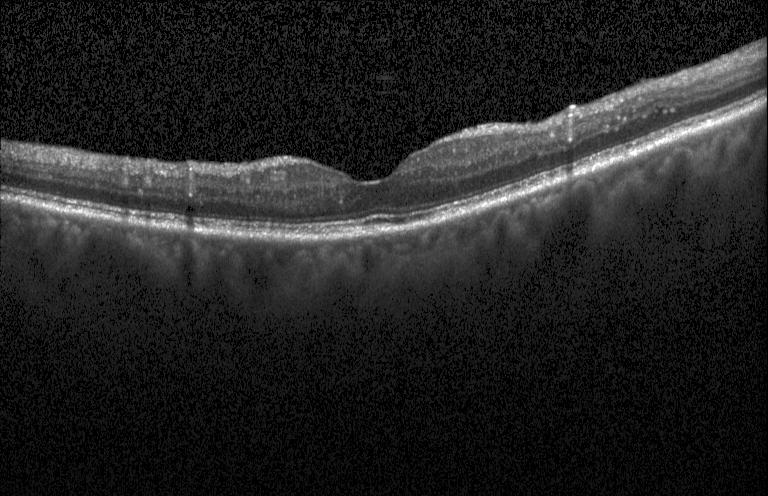

OCT line scan.
This B-scan demonstrates neither choroidal neovascularization, diabetic macular edema, nor drusen.